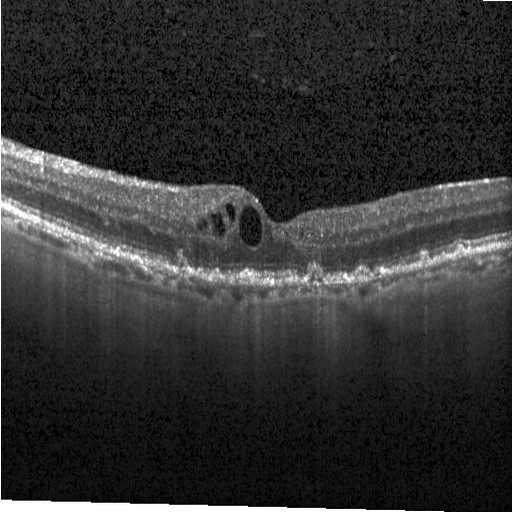

Retinal OCT cross-section
Finding: diabetic macular edema.